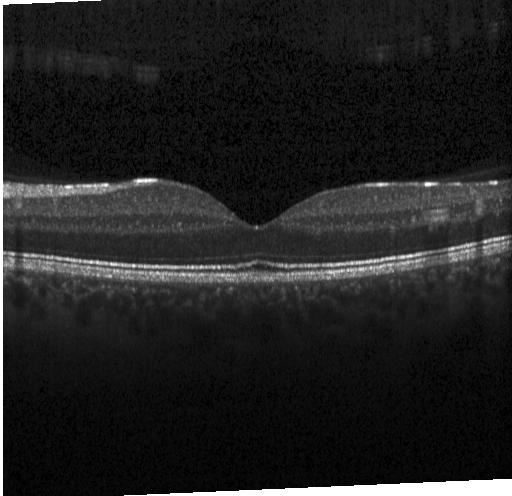

SD-OCT, Heidelberg Spectralis OCT system, OCT B-scan
Finding: no CNV, DME, or drusen.